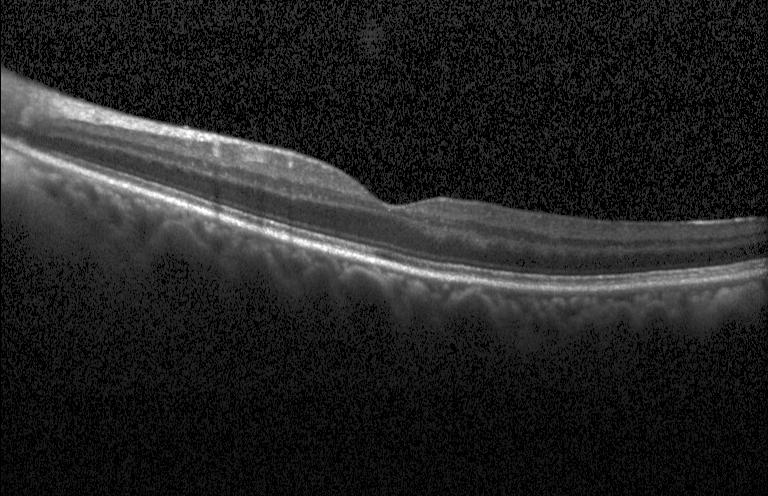 Impression: no choroidal neovascularization, no diabetic macular edema, and no drusen.